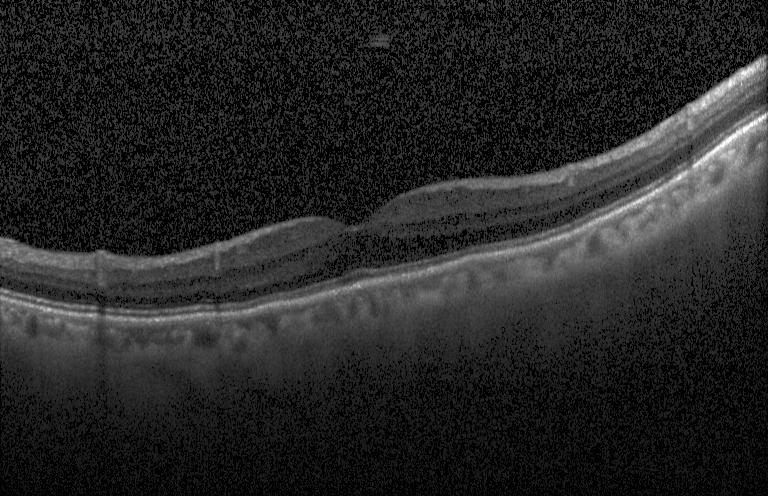 The scan shows no evidence of CNV, DME, or drusen.